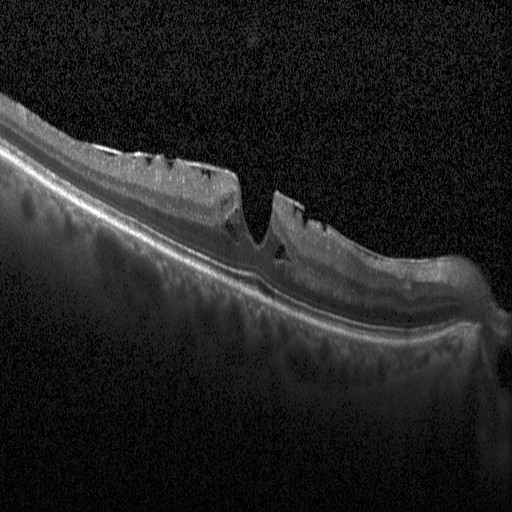

Heidelberg Spectralis OCT system, OCT line scan, spectral-domain OCT.
Finding: DME.